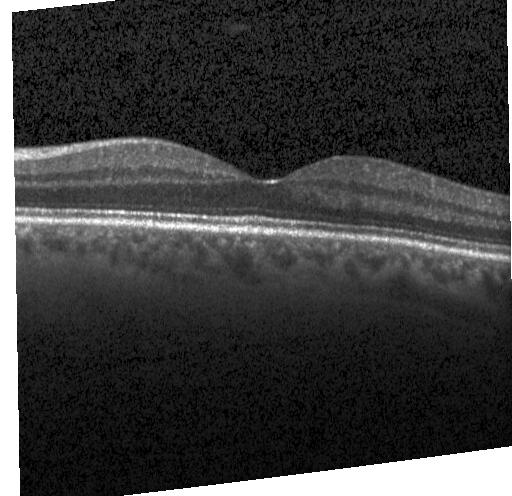
Through the macula. Optical coherence tomography B-scan. Heidelberg Spectralis OCT system
Diagnosis: neither choroidal neovascularization, diabetic macular edema, nor drusen.